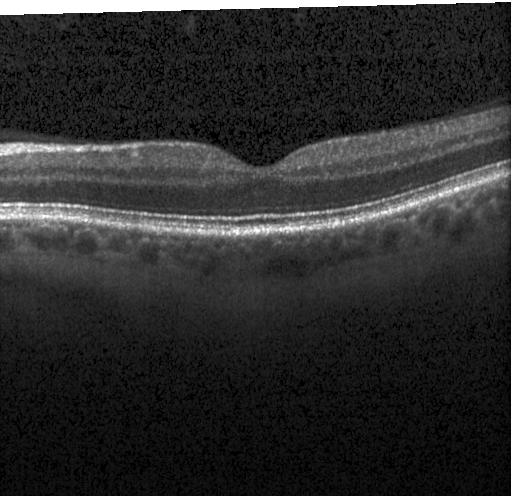

Optical coherence tomography scan.
Diagnosis: no choroidal neovascularization, diabetic macular edema, or drusen.